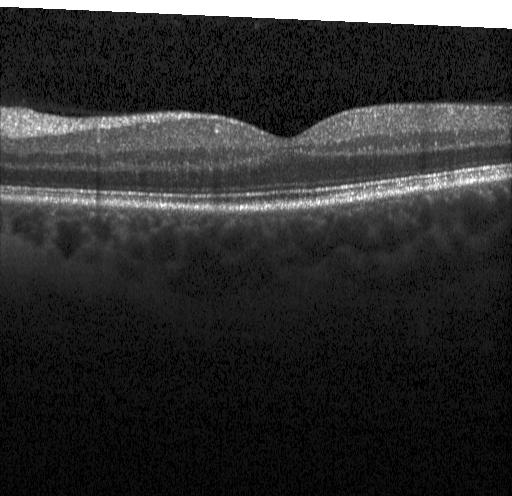
OCT line scan; spectral-domain optical coherence tomography — Impression: neither choroidal neovascularization, diabetic macular edema, nor drusen.